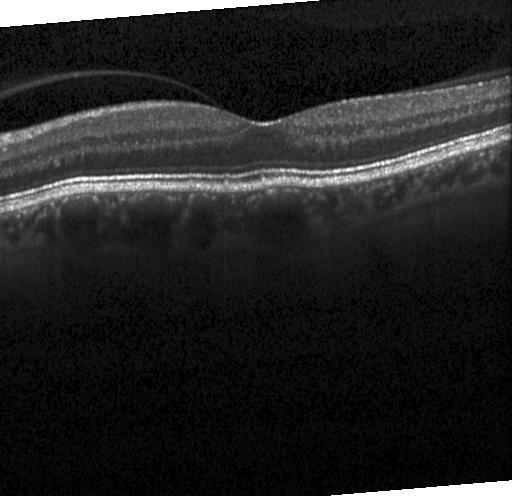
Diagnosis: no evidence of CNV, DME, or drusen.